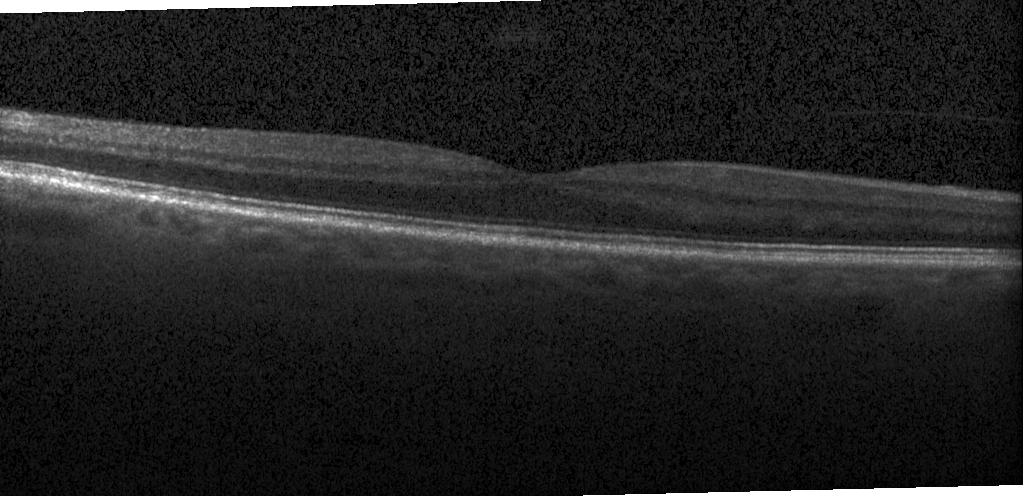 The scan shows no evidence of CNV, DME, or drusen.